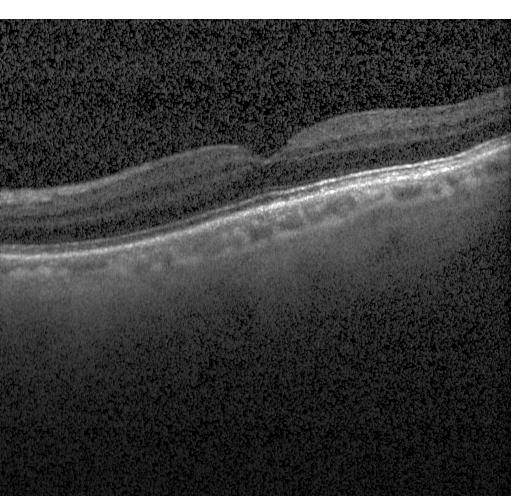 Spectral-domain OCT, instrument: Heidelberg Spectralis, through the macula, optical coherence tomography scan.
Assessment: no choroidal neovascularization, no diabetic macular edema, and no drusen.